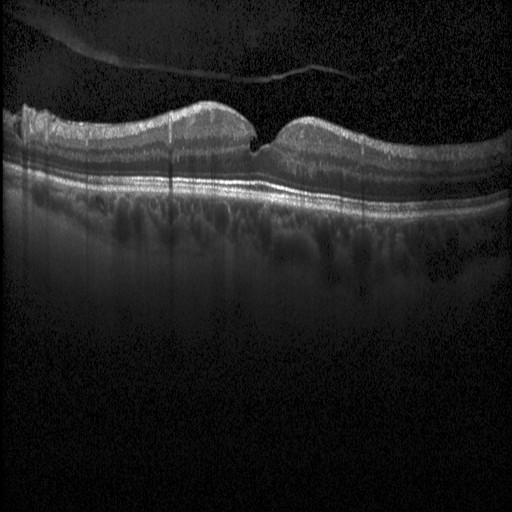
OCT line scan — Dx: diabetic macular edema (DME).